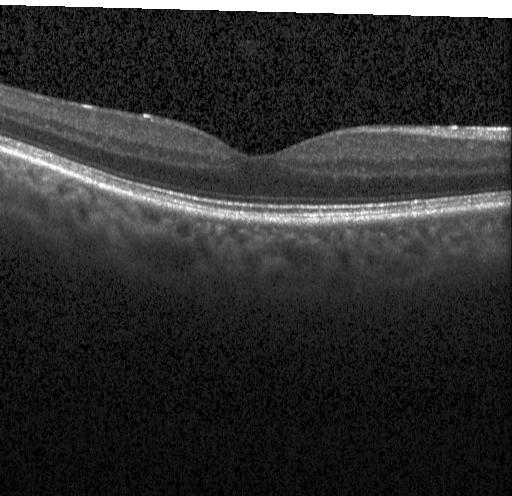
Dx: no choroidal neovascularization, no diabetic macular edema, and no drusen.